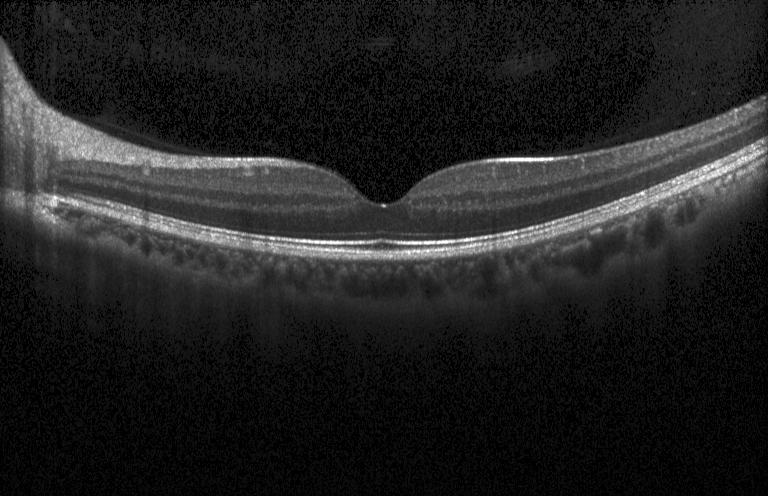 This B-scan demonstrates no choroidal neovascularization, no diabetic macular edema, and no drusen.